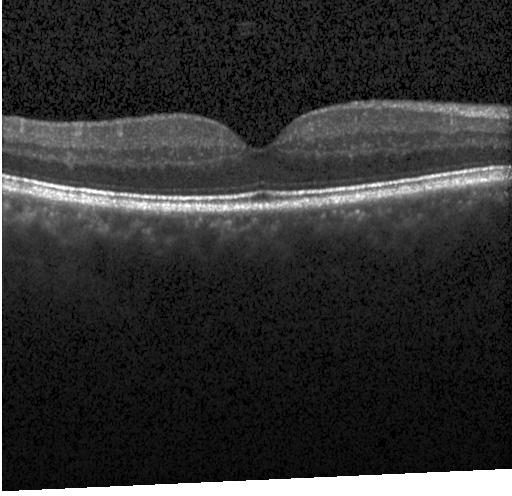
Retinal OCT B-scan
Diagnosis: no CNV, DME, or drusen.